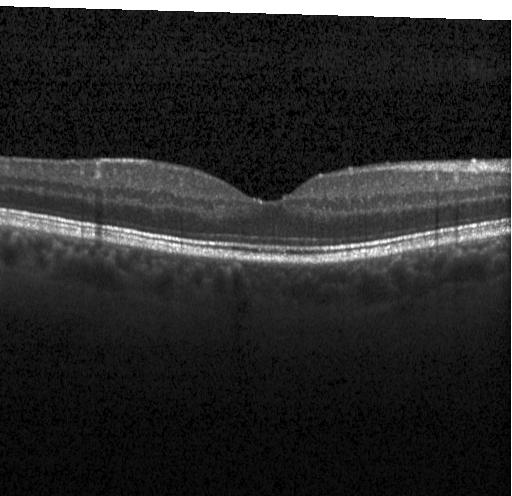 Optical coherence tomography B-scan; Heidelberg Spectralis; macular scan — Diagnosis: no choroidal neovascularization, diabetic macular edema, or drusen.